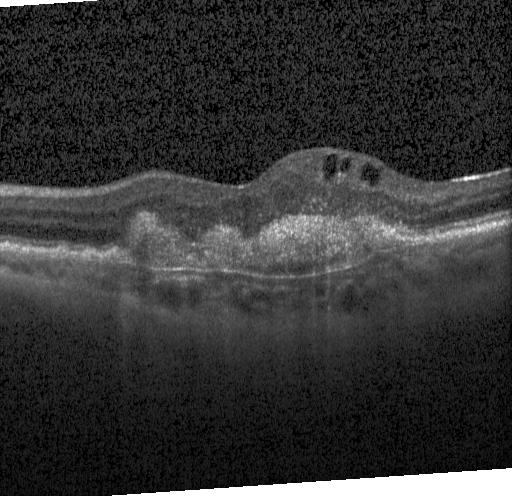 Acquired on a Heidelberg Spectralis, horizontal scan through the fovea, SD-OCT, retinal OCT B-scan — The scan shows a choroidal neovascular membrane.